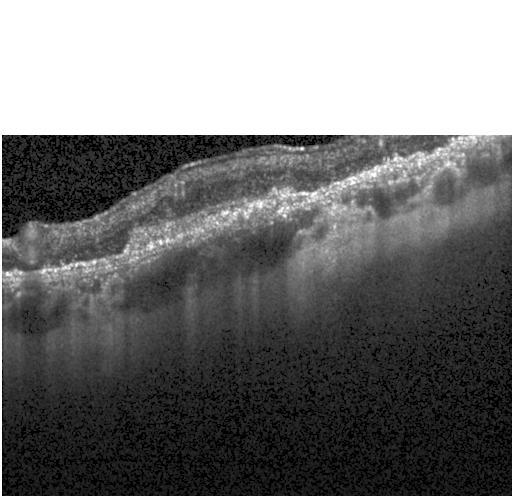

OCT scan showing a choroidal neovascular membrane.